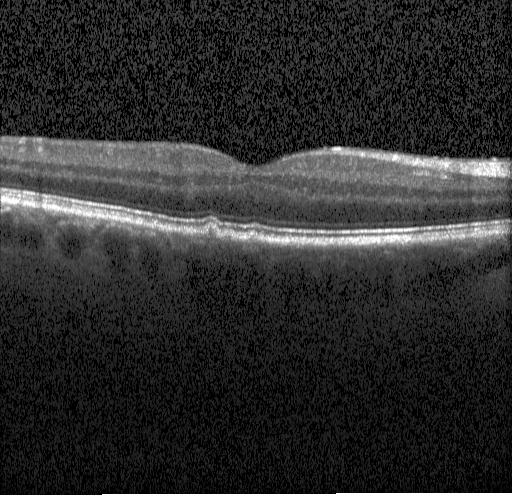
Centered on the fovea; retinal OCT cross-section — Impression: sub-RPE drusenoid deposits.